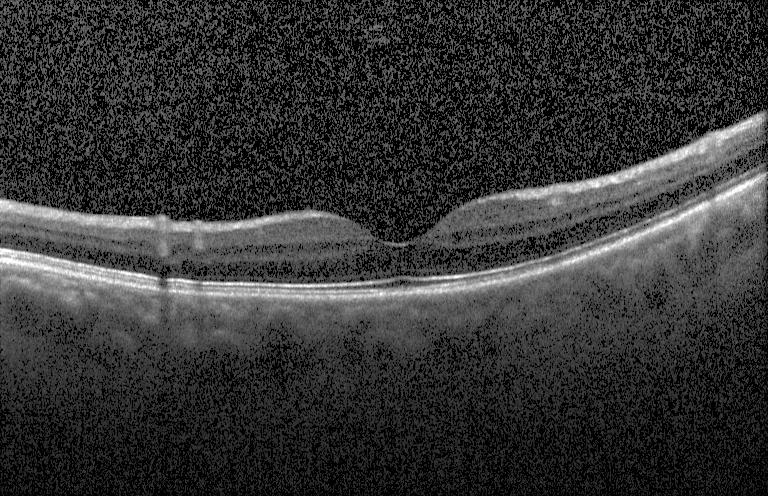

Through the macula; Heidelberg Spectralis; optical coherence tomography scan.
Impression: no choroidal neovascularization, no diabetic macular edema, and no drusen.